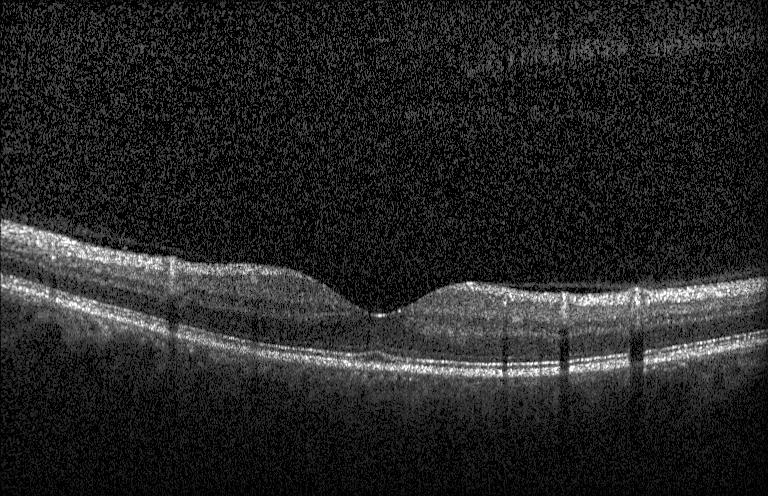
Spectral-domain optical coherence tomography. Optical coherence tomography B-scan. Fovea-centered.
Finding: no evidence of CNV, DME, or drusen.